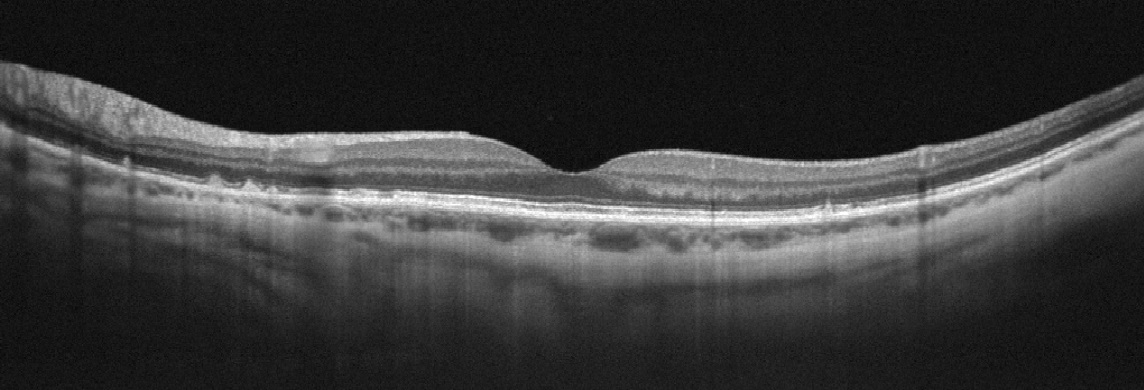 Dx: age-related macular degeneration (AMD).